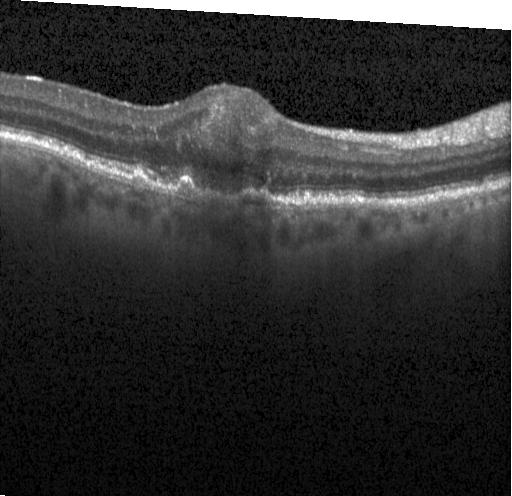

Retinal OCT cross-section.
Diagnosis: choroidal neovascularization.